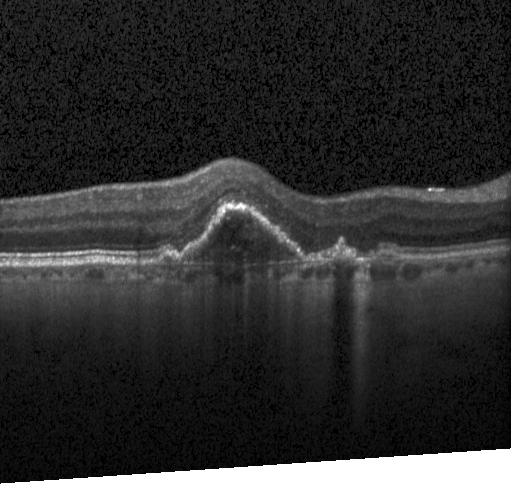
OCT line scan — This B-scan demonstrates CNV.